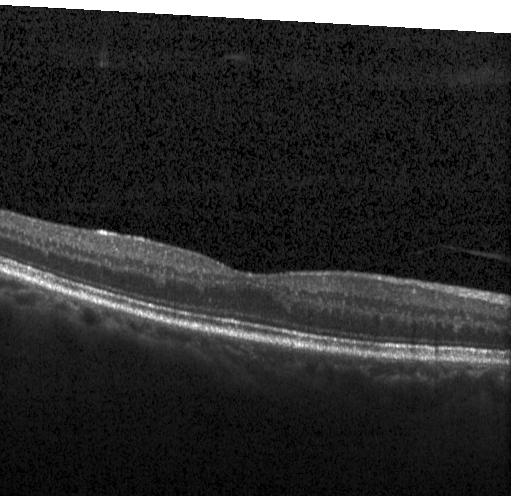
Neither CNV, DME, nor drusen.